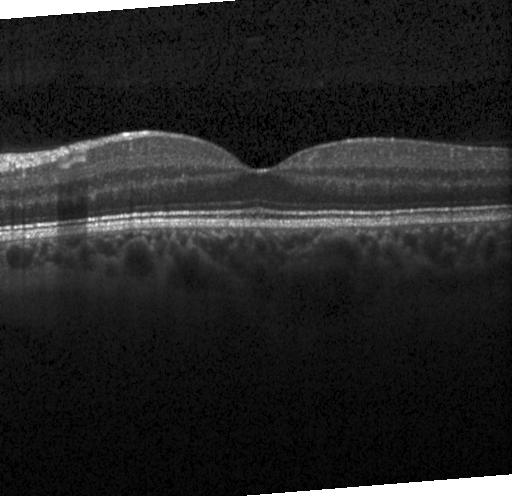
OCT line scan
No evidence of choroidal neovascularization, diabetic macular edema, or drusen.